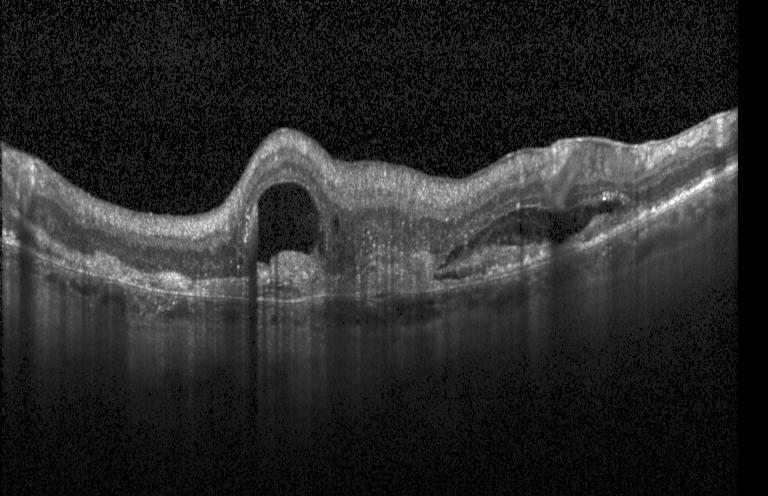

Through the macula; spectral-domain optical coherence tomography; acquired on a Heidelberg Spectralis; OCT B-scan.
Diagnosis: choroidal neovascularization (CNV).